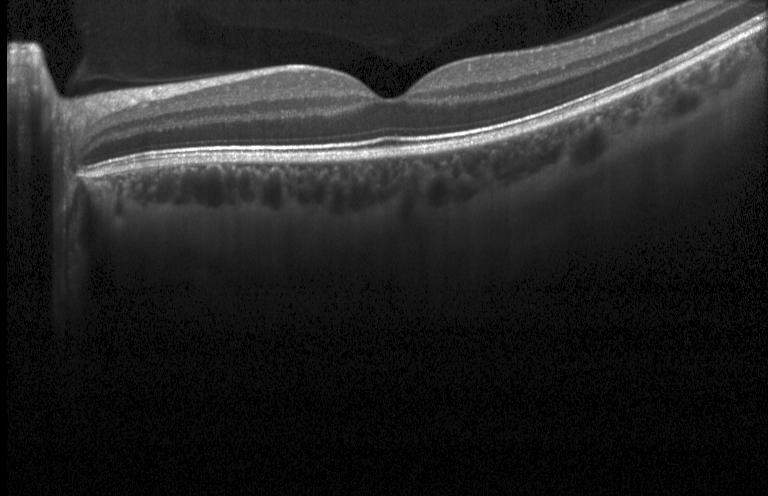

Spectral-domain optical coherence tomography; macular scan; retinal OCT cross-section; instrument: Heidelberg Spectralis — Diagnosis: no choroidal neovascularization, no diabetic macular edema, and no drusen.